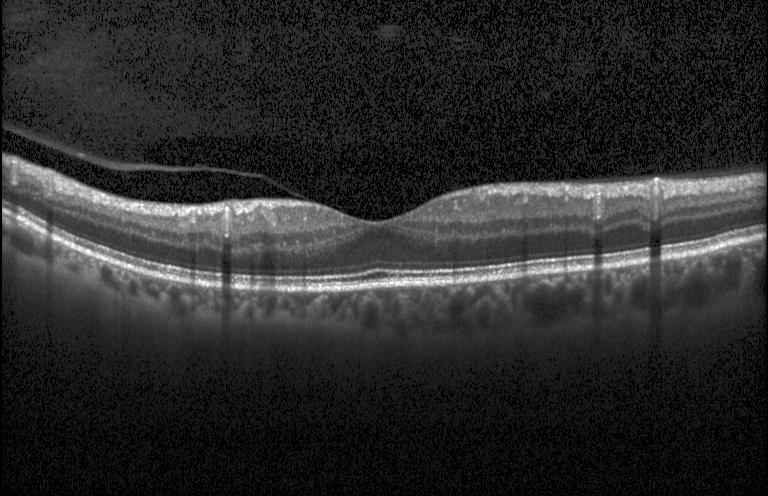 Spectral-domain OCT B-scan: no CNV, no DME, and no drusen.